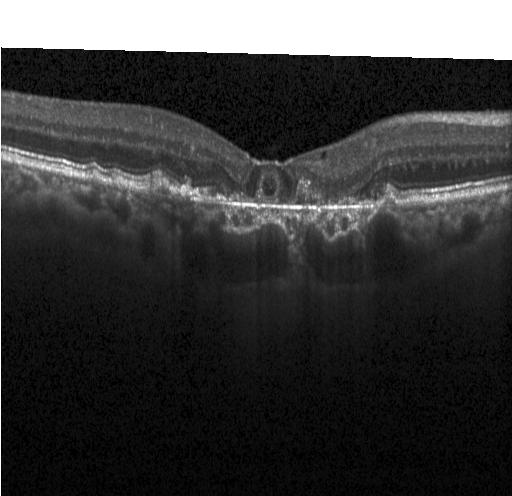
Diagnosis: choroidal neovascularization (CNV).